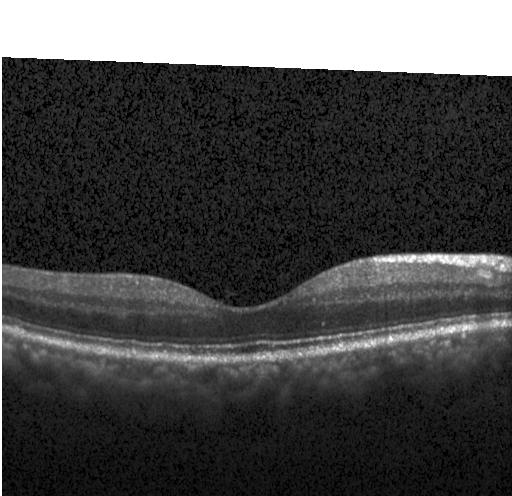

Optical coherence tomography scan
Dx: no choroidal neovascularization, diabetic macular edema, or drusen.